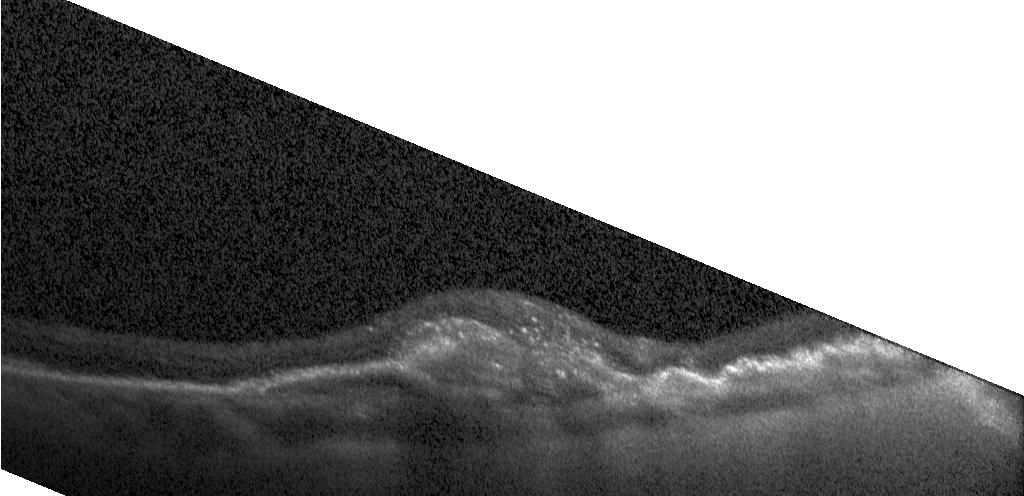 Impression: CNV.